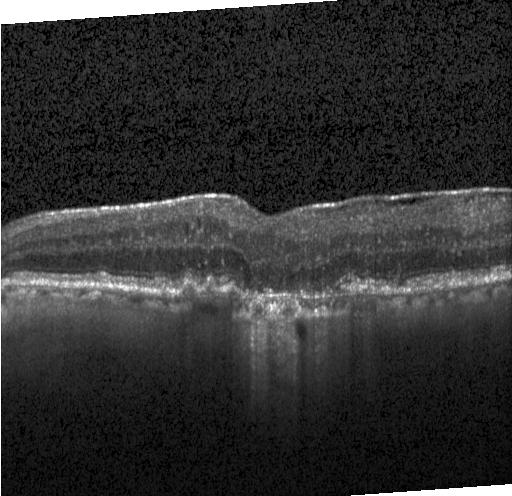 Retinal OCT cross-section — Diagnosis: choroidal neovascularization (CNV).